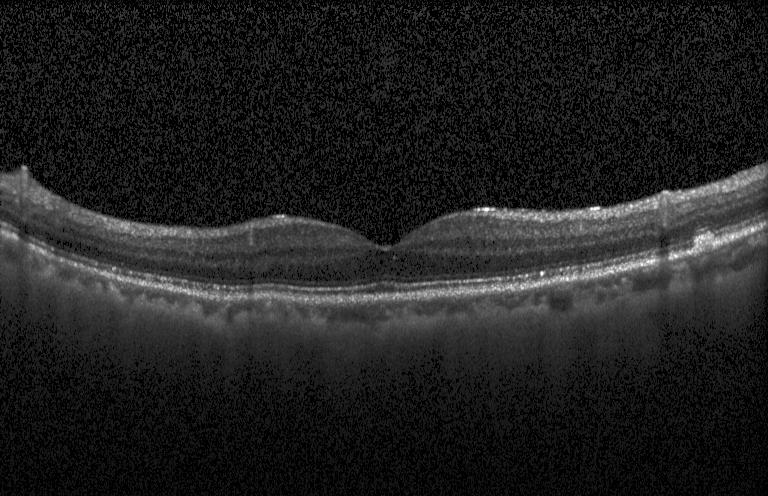
Spectral-domain OCT. Heidelberg Spectralis OCT system. Retinal OCT B-scan. Macular scan
Diagnosis: drusen.